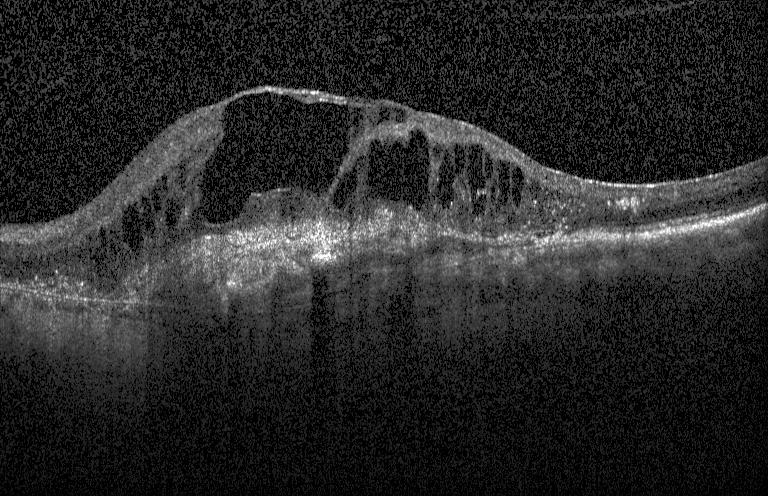
Optical coherence tomography B-scan — Finding: a choroidal neovascular membrane.